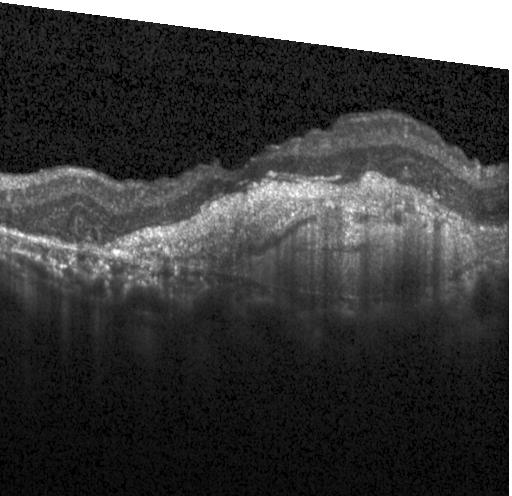
SD-OCT · Heidelberg Spectralis OCT system · optical coherence tomography B-scan · macular scan.
Impression: choroidal neovascularization (CNV).